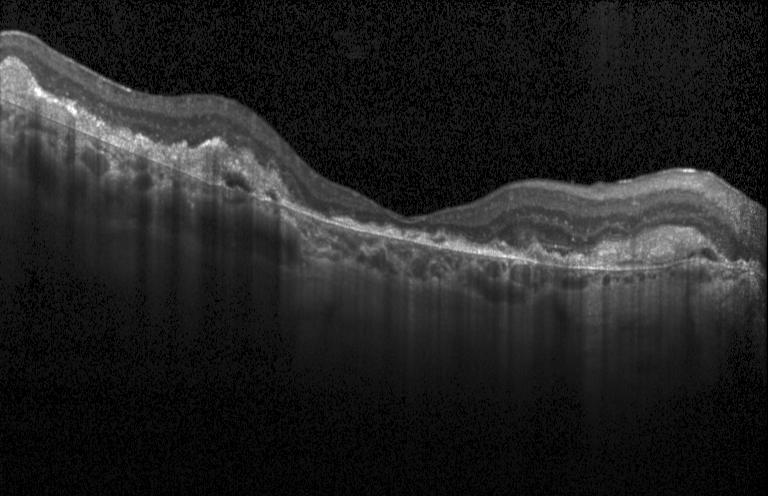
Dx: a choroidal neovascular membrane.